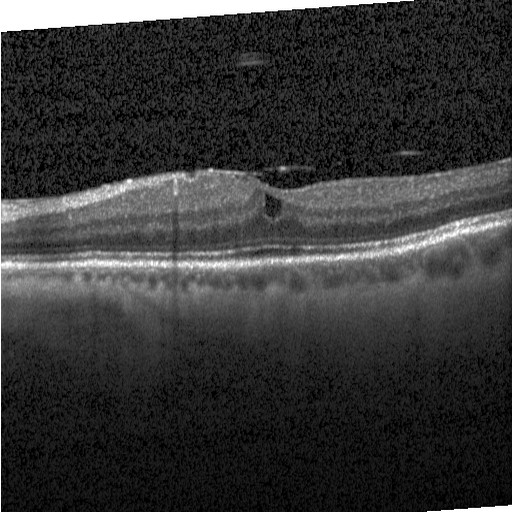
Centered on the fovea; spectral-domain optical coherence tomography; optical coherence tomography scan; acquired on a Heidelberg Spectralis. The scan shows DME.